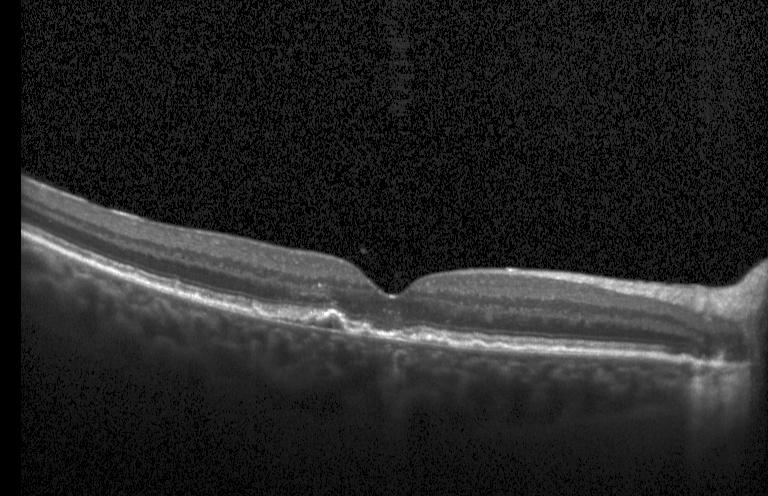

Retinal OCT cross-section. Fovea-centered. Spectral-domain optical coherence tomography. Acquired on a Heidelberg Spectralis
Macular OCT: multiple drusen.